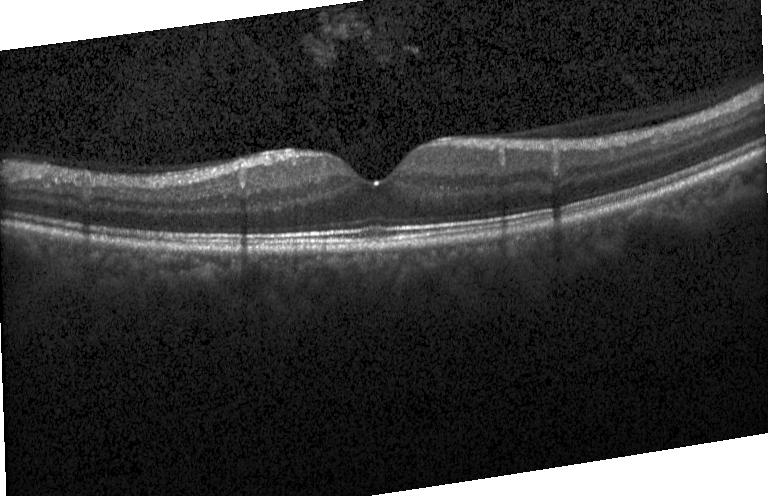

Finding: no choroidal neovascularization, no diabetic macular edema, and no drusen.